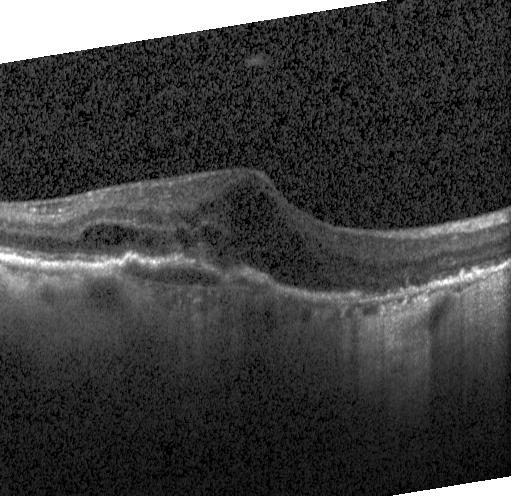

OCT line scan — Finding: a choroidal neovascular membrane.